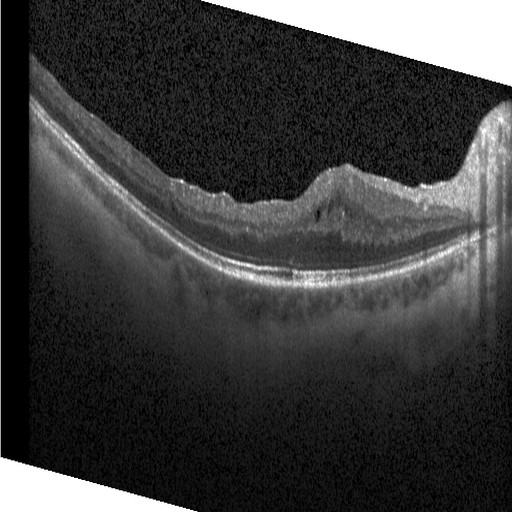 Diabetic macular edema.